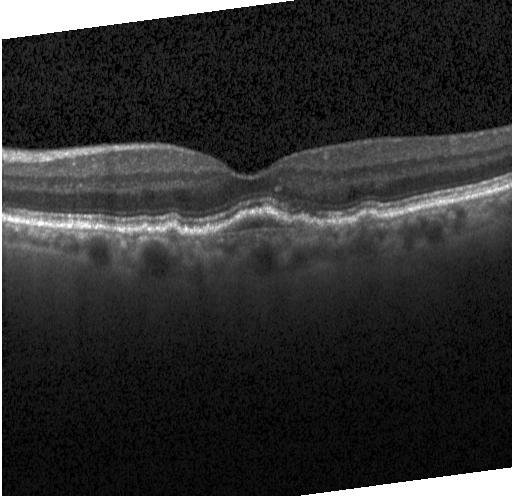
A choroidal neovascular membrane.